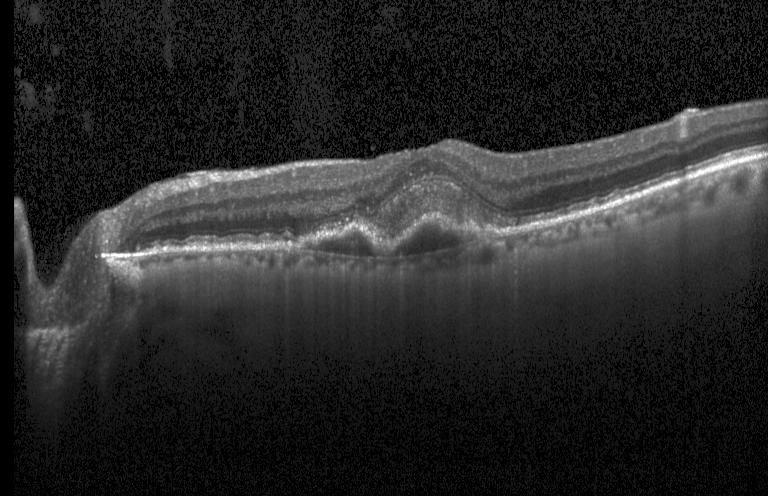
Optical coherence tomography scan.
Diagnosis: a choroidal neovascular membrane.